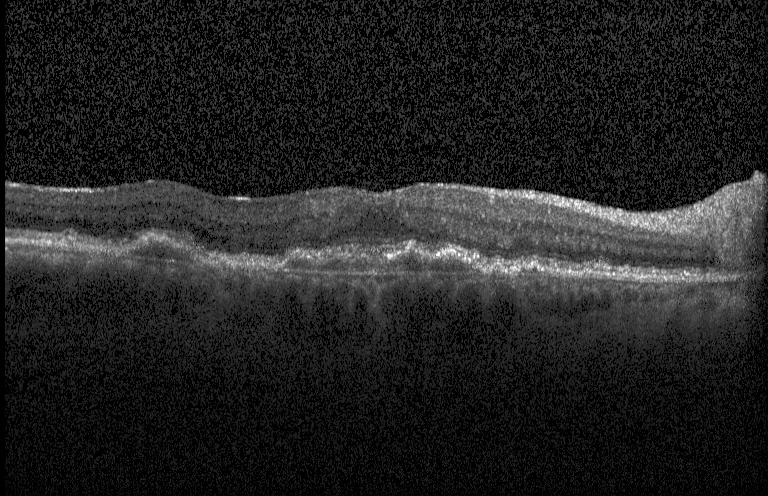

Optical coherence tomography scan, macular scan.
Impression: CNV.